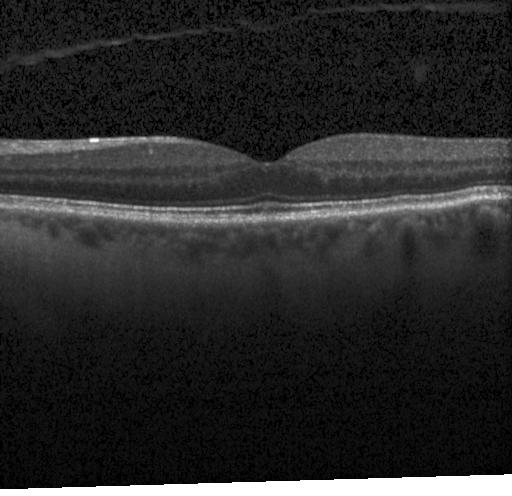

Optical coherence tomography scan · spectral-domain OCT · acquired on a Heidelberg Spectralis — Finding: no CNV, DME, or drusen.